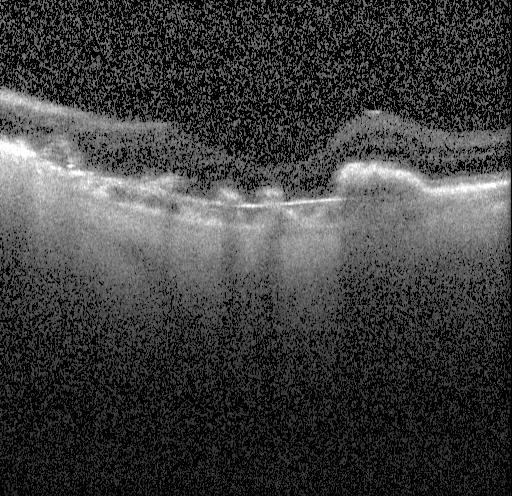

Retinal OCT cross-section showing a choroidal neovascular membrane.